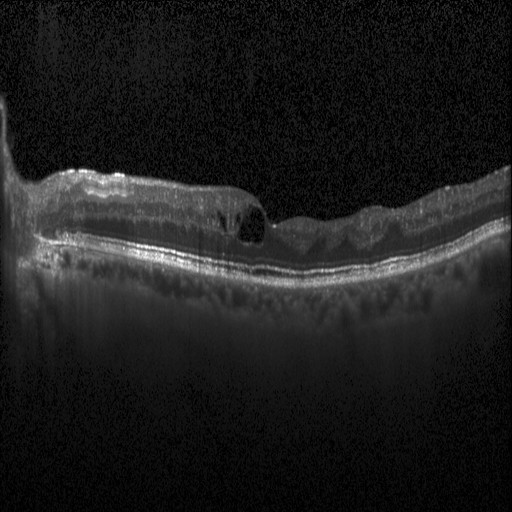

OCT B-scan. This B-scan demonstrates diabetic macular edema.